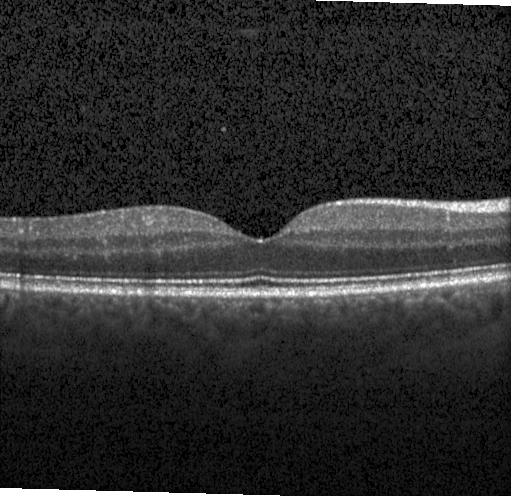
Macular scan; optical coherence tomography scan. Diagnosis: neither choroidal neovascularization, diabetic macular edema, nor drusen.